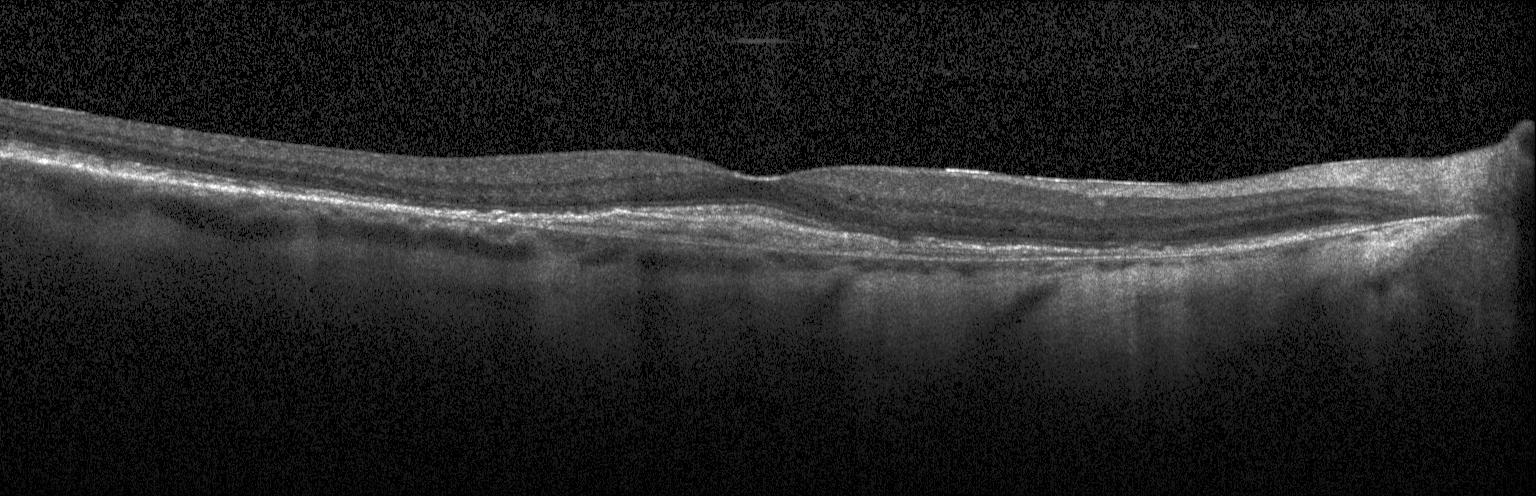
Retinal OCT B-scan, SD-OCT.
Finding: CNV.